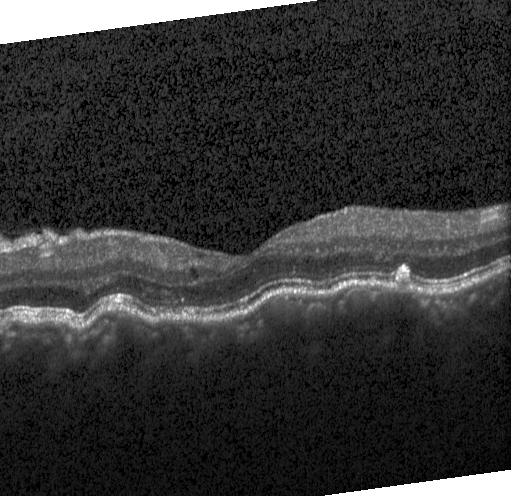
Through the macula. Optical coherence tomography B-scan. Heidelberg Spectralis OCT system. SD-OCT. Diagnosis: multiple drusen.